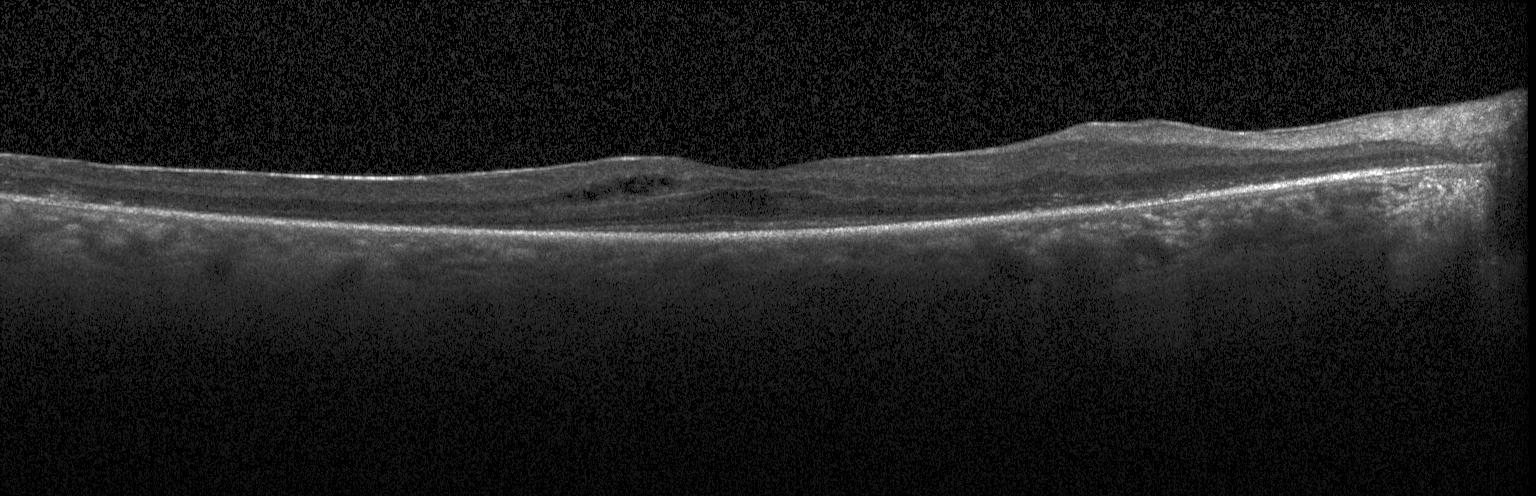

Finding: diabetic macular edema (DME).